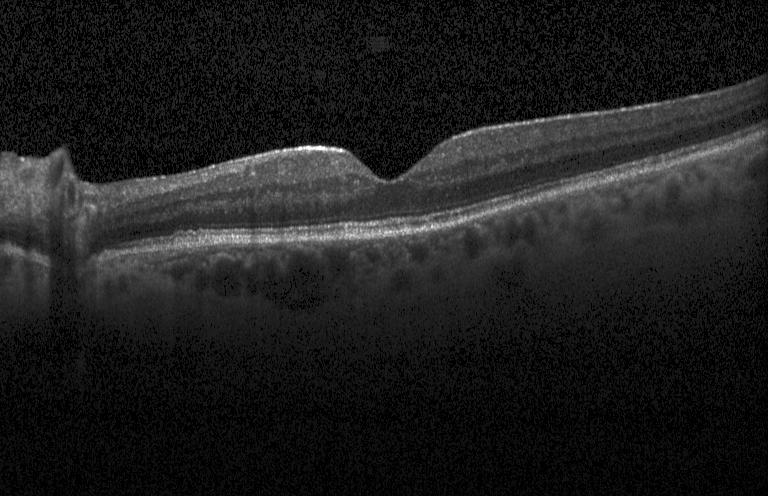

Optical coherence tomography scan · Heidelberg Spectralis · spectral-domain OCT
Finding: no choroidal neovascularization, no diabetic macular edema, and no drusen.